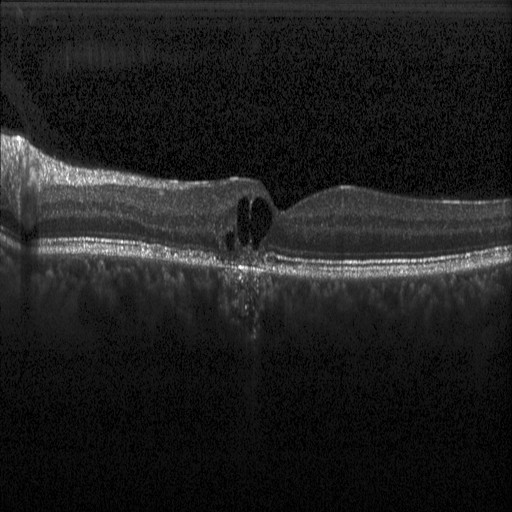 Optical coherence tomography scan — Diagnosis: diabetic macular edema.